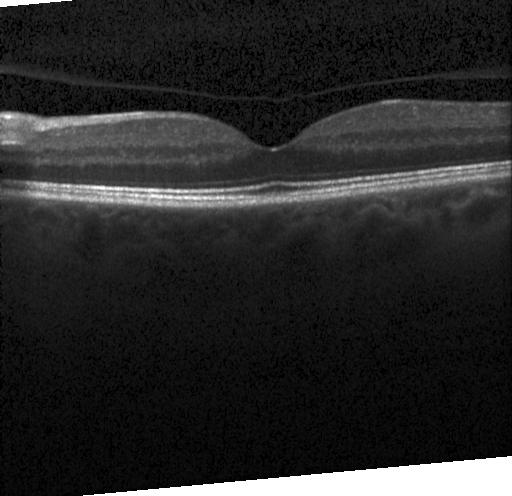

Spectral-domain OCT; optical coherence tomography B-scan; centered on the fovea; acquired on a Heidelberg Spectralis. Assessment: neither choroidal neovascularization, diabetic macular edema, nor drusen.